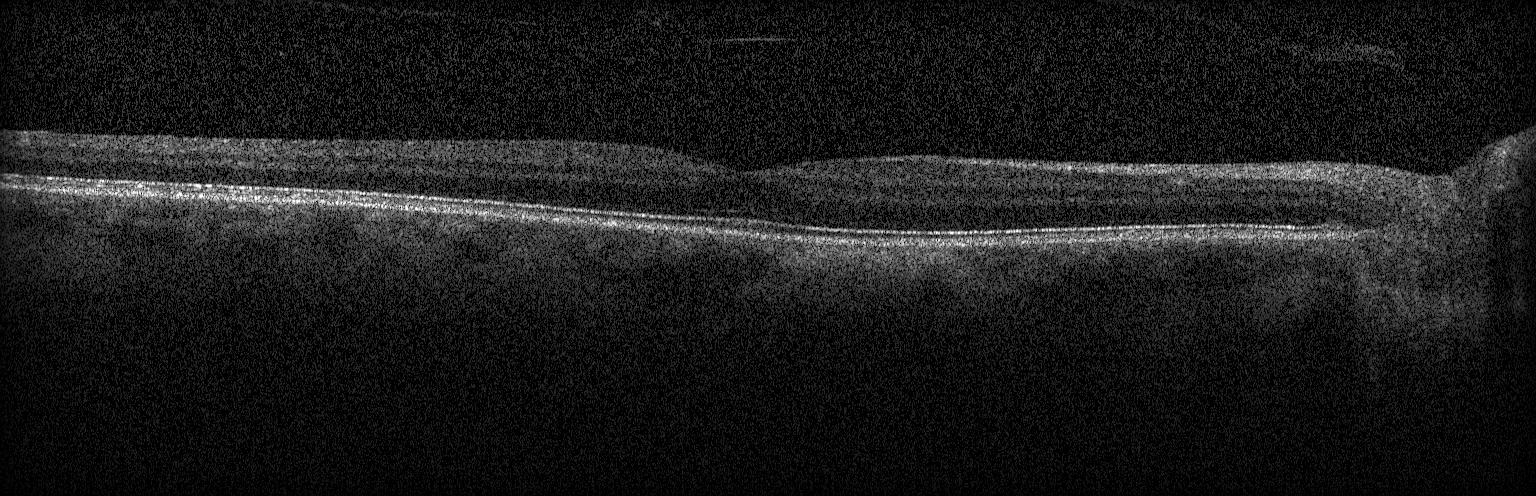
OCT finding: neither choroidal neovascularization, diabetic macular edema, nor drusen.